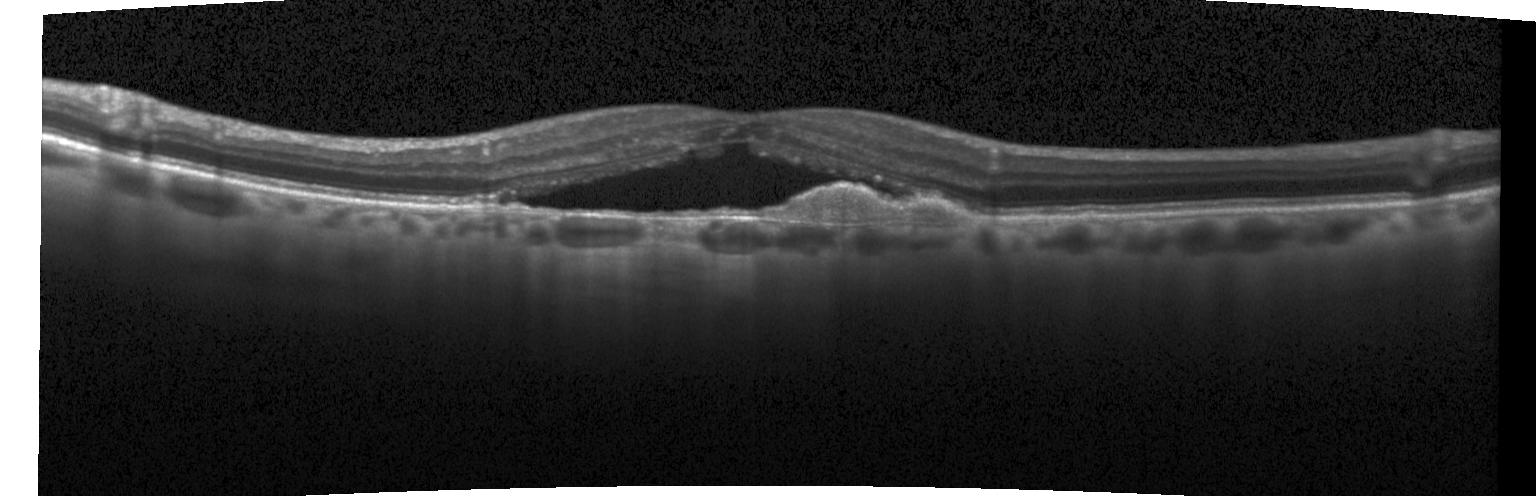
The scan shows a choroidal neovascular membrane.